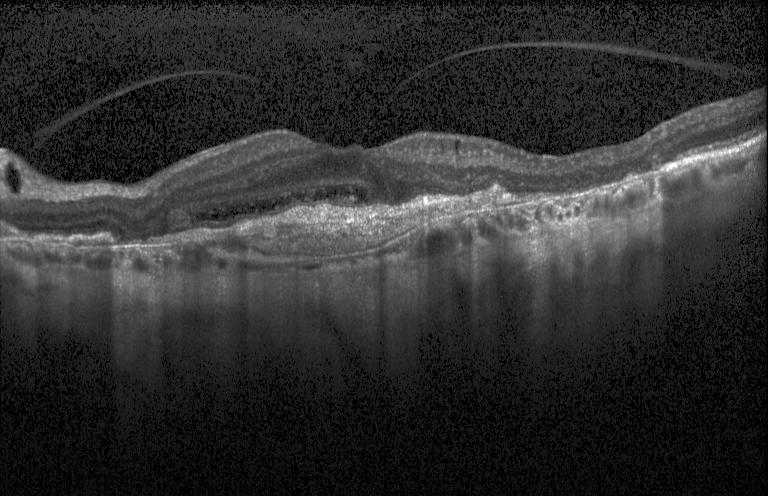

Through the macula · OCT line scan · Heidelberg Spectralis OCT system · SD-OCT — Assessment: a choroidal neovascular membrane.